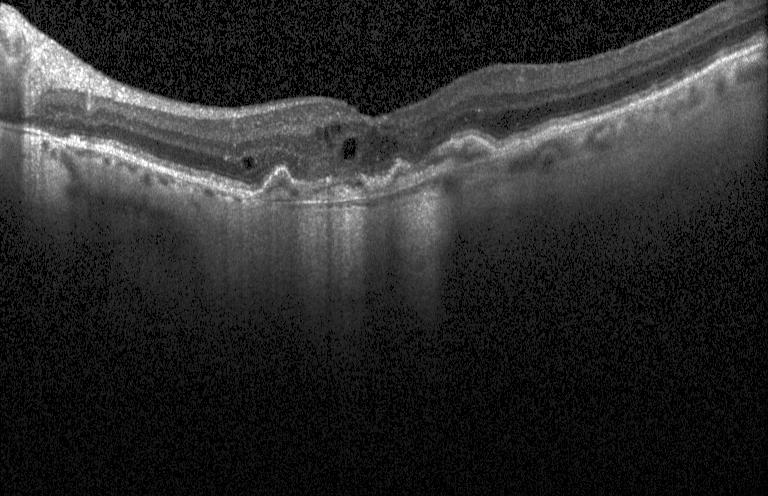
OCT line scan
Macular OCT: a choroidal neovascular membrane.